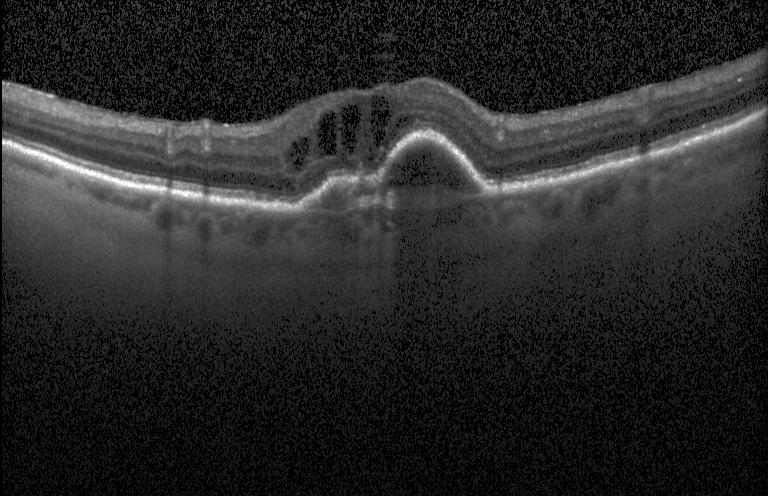

Acquired on a Heidelberg Spectralis. Retinal OCT cross-section.
Choroidal neovascularization.